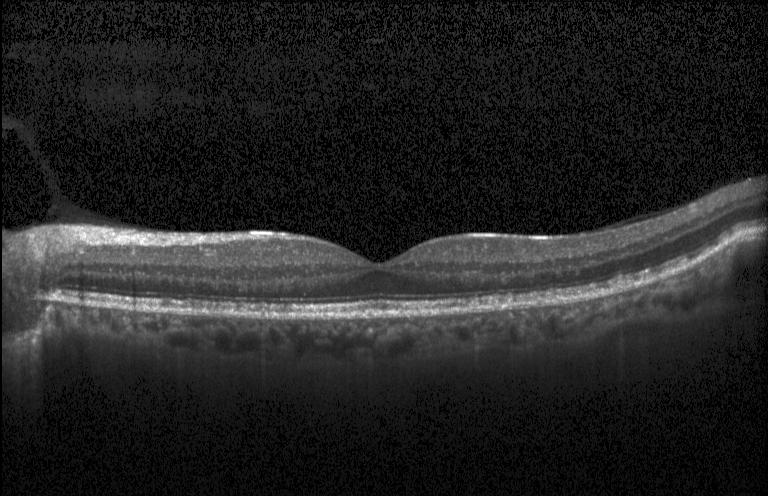 Retinal OCT cross-section, SD-OCT, through the macula.
The scan shows neither choroidal neovascularization, diabetic macular edema, nor drusen.